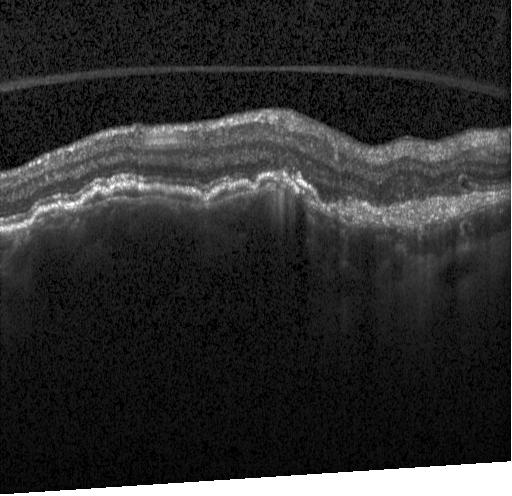
Retinal OCT B-scan, Heidelberg Spectralis
Finding: choroidal neovascularization.